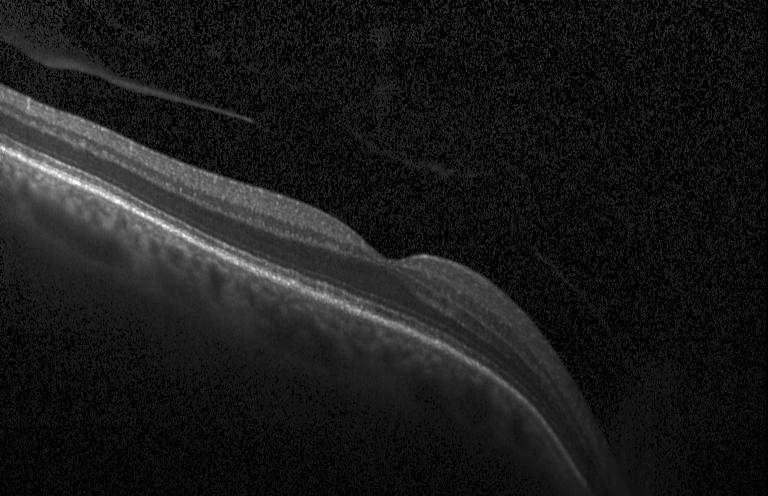 Acquired on a Heidelberg Spectralis, OCT B-scan, SD-OCT.
Impression: neither CNV, DME, nor drusen.